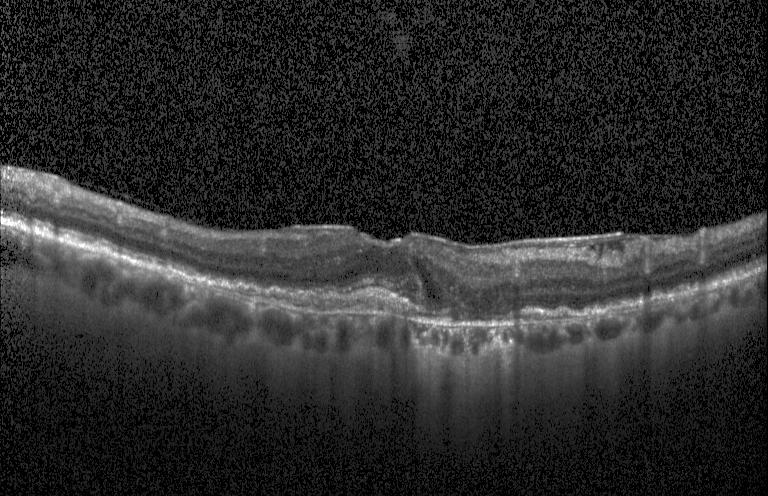 OCT line scan · horizontal scan through the fovea · Heidelberg Spectralis OCT system
Finding: a choroidal neovascular membrane.